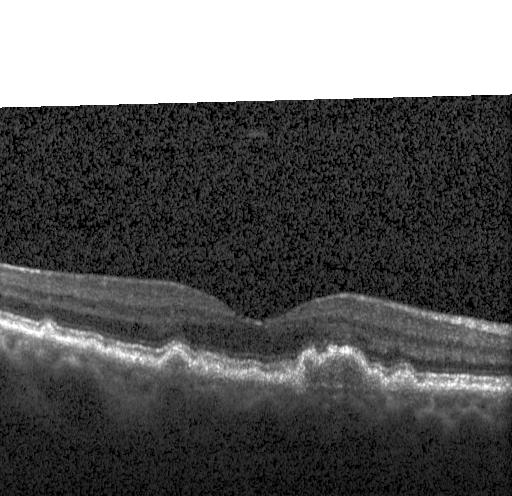 Optical coherence tomography B-scan · instrument: Heidelberg Spectralis · macular scan · spectral-domain OCT. The scan shows sub-RPE drusenoid deposits.